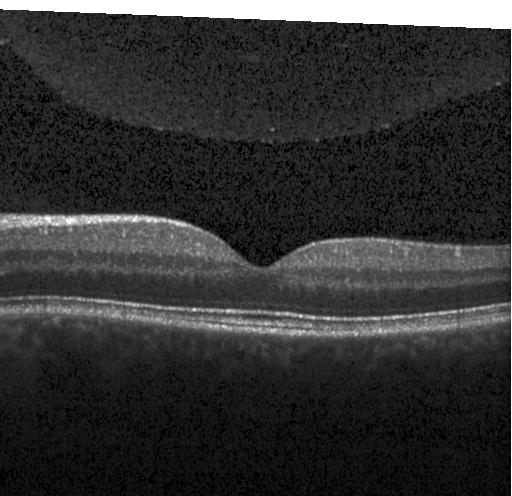

OCT scan showing no evidence of choroidal neovascularization, diabetic macular edema, or drusen.